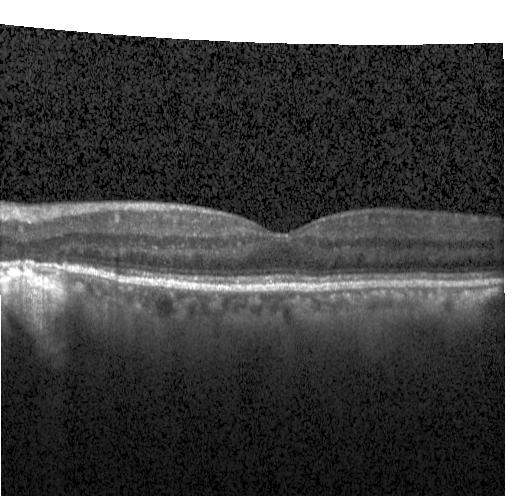

OCT finding: no evidence of choroidal neovascularization, diabetic macular edema, or drusen.